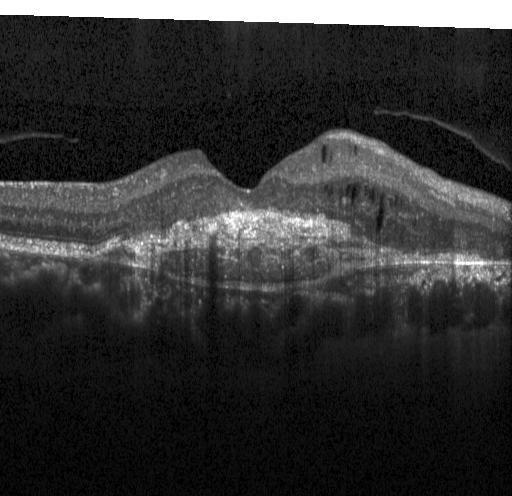 Retinal OCT cross-section. Spectral-domain optical coherence tomography — This B-scan demonstrates choroidal neovascularization.